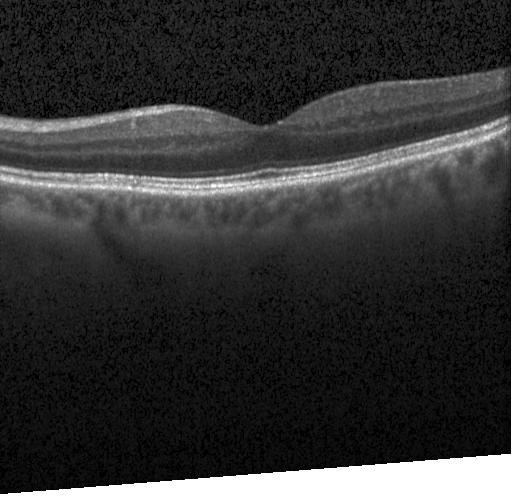

OCT B-scan — Dx: no choroidal neovascularization, diabetic macular edema, or drusen.